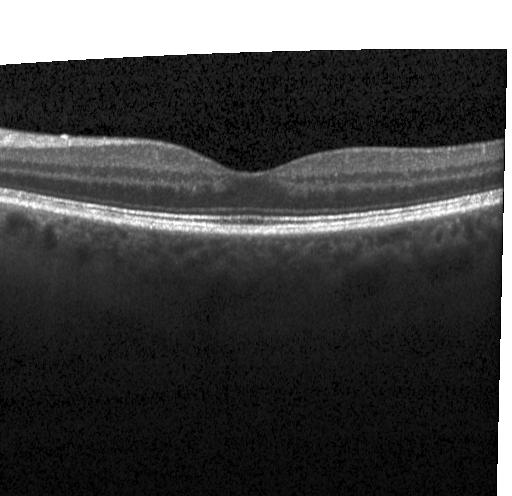

Retinal OCT B-scan. Fovea-centered. Heidelberg Spectralis OCT system. SD-OCT.
The scan shows no evidence of CNV, DME, or drusen.